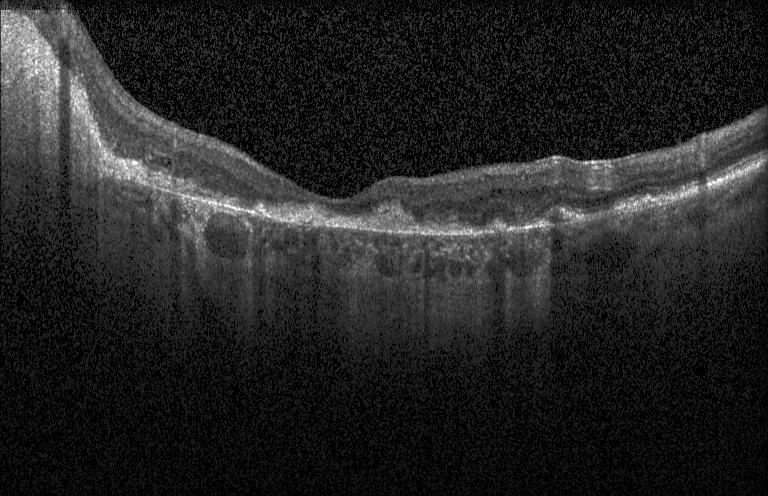 OCT B-scan showing CNV.